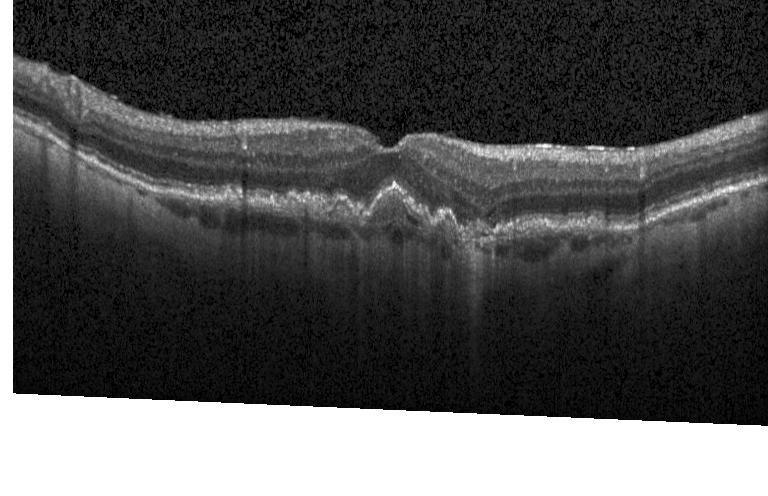
Finding: CNV.